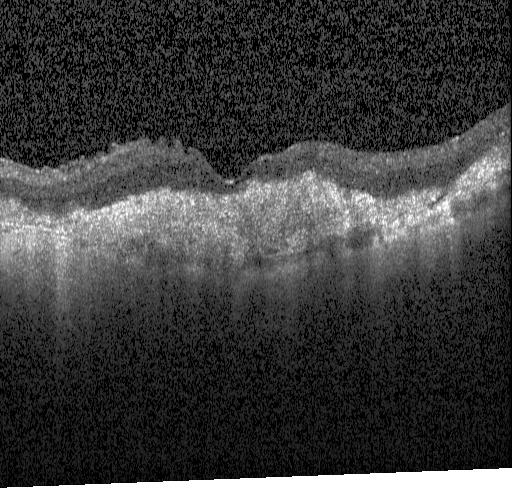
Spectral-domain OCT B-scan: a choroidal neovascular membrane.